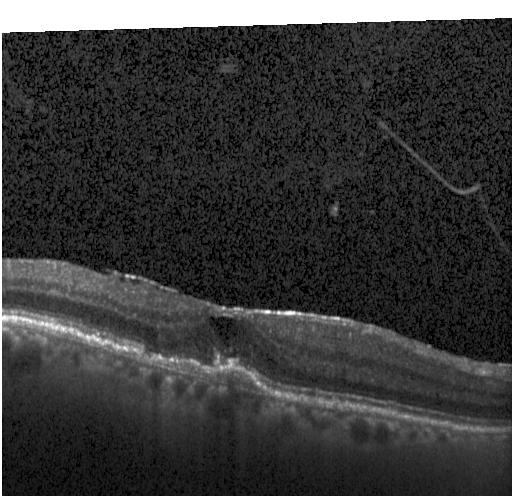

Macular OCT: choroidal neovascularization (CNV).